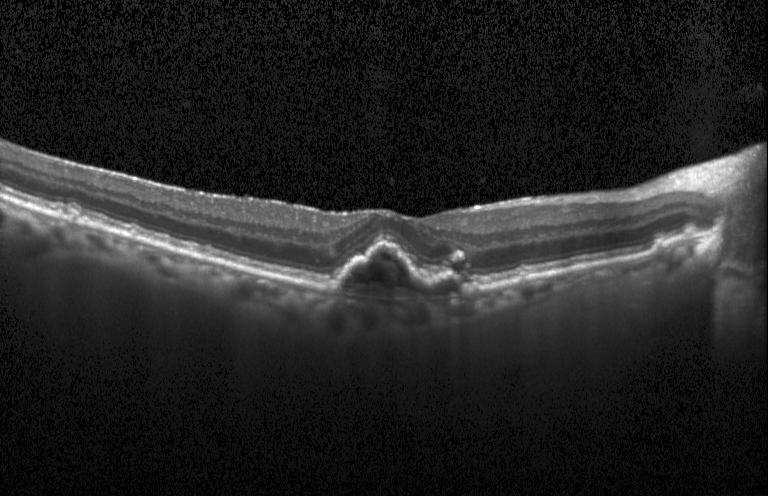

OCT B-scan — Finding: a choroidal neovascular membrane.